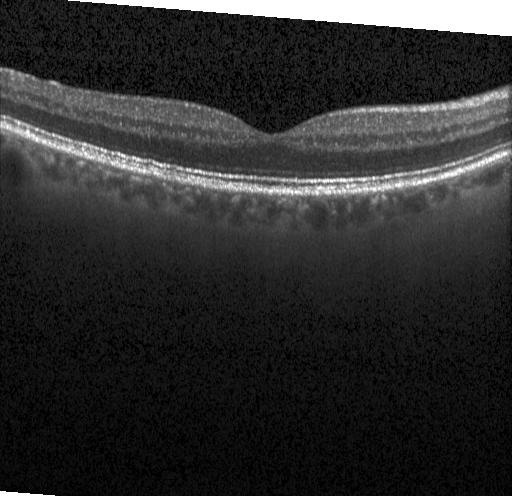

OCT line scan. Diagnosis: no evidence of choroidal neovascularization, diabetic macular edema, or drusen.